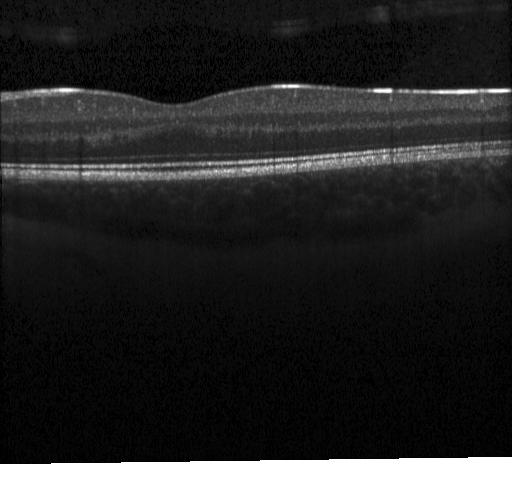

OCT B-scan.
No choroidal neovascularization, no diabetic macular edema, and no drusen.